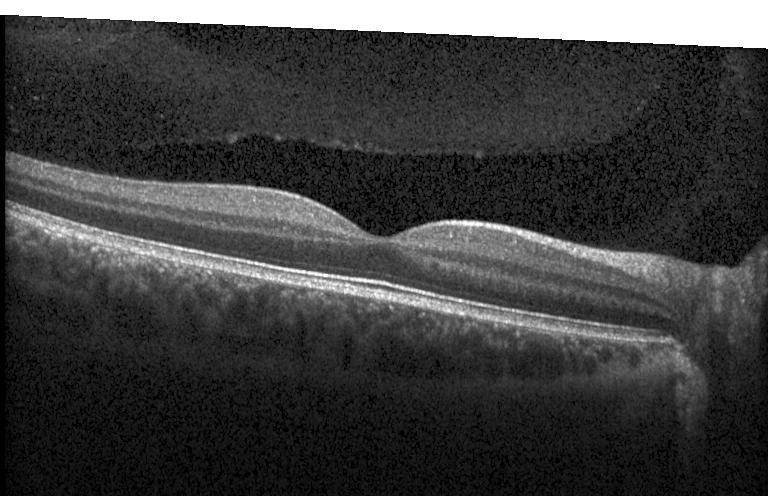
Diagnosis: no CNV, DME, or drusen.